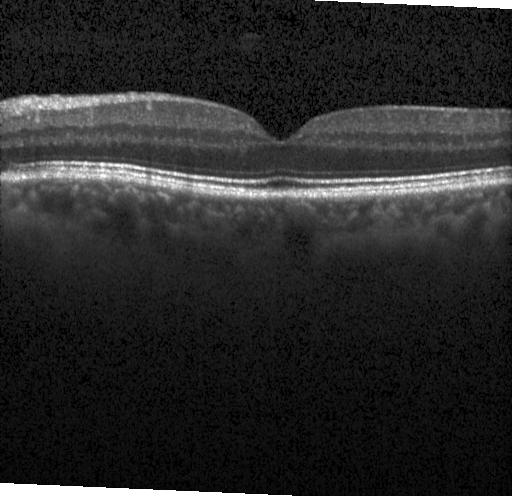 Impression: no choroidal neovascularization, no diabetic macular edema, and no drusen.